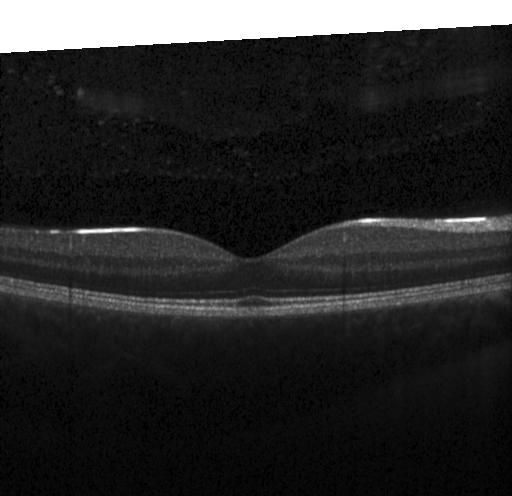 OCT B-scan, centered on the fovea, Heidelberg Spectralis
Finding: no choroidal neovascularization, no diabetic macular edema, and no drusen.